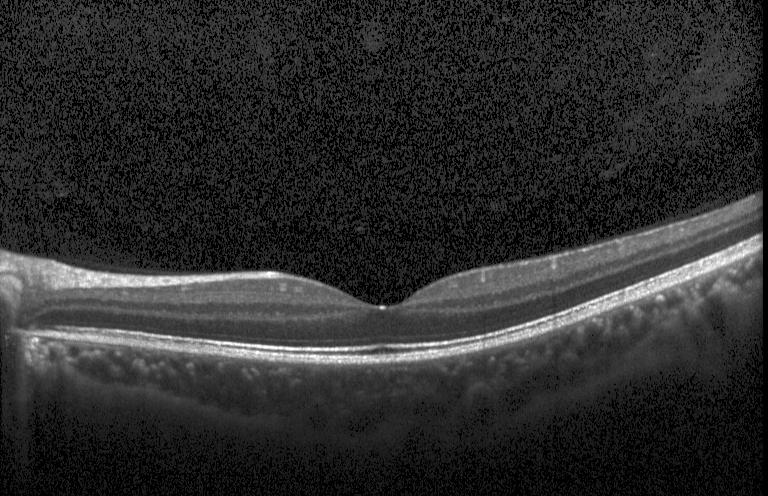

Optical coherence tomography scan. Acquired on a Heidelberg Spectralis. Spectral-domain optical coherence tomography.
Finding: no choroidal neovascularization, no diabetic macular edema, and no drusen.